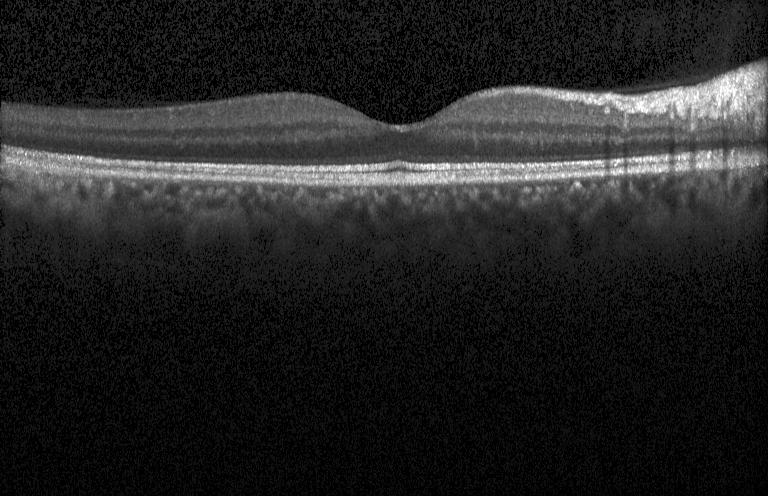
Retinal OCT B-scan, fovea-centered, instrument: Heidelberg Spectralis — Finding: no choroidal neovascularization, diabetic macular edema, or drusen.